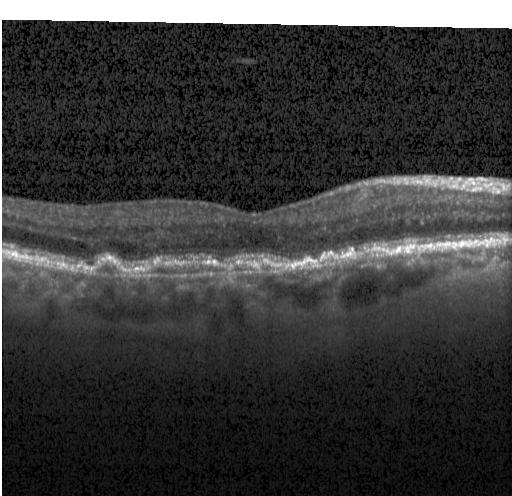

Impression: a choroidal neovascular membrane.